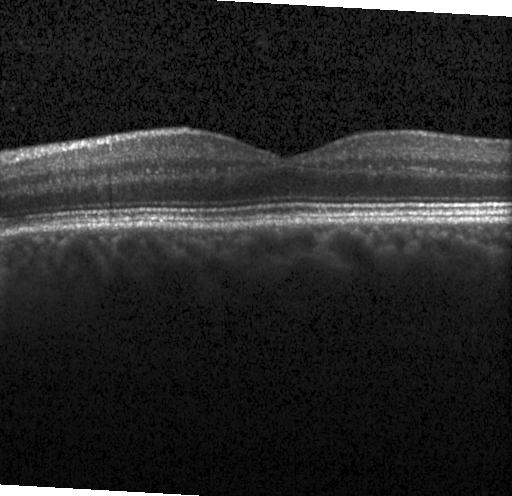

Macular scan; instrument: Heidelberg Spectralis; OCT B-scan — This B-scan demonstrates no choroidal neovascularization, no diabetic macular edema, and no drusen.